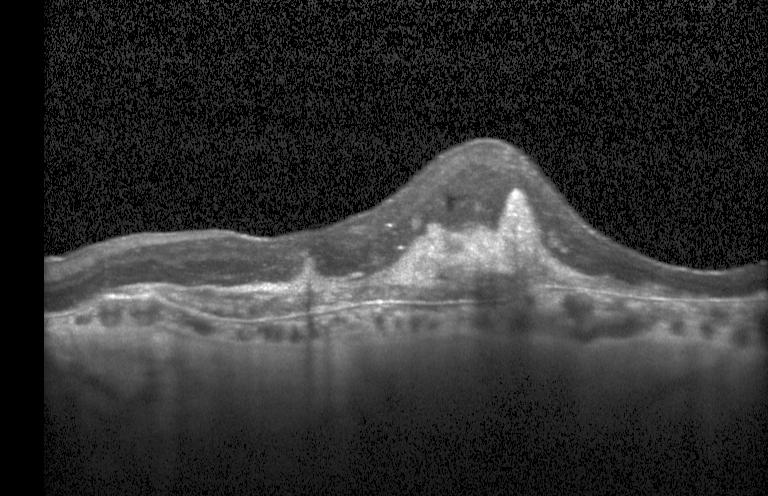
Choroidal neovascularization.